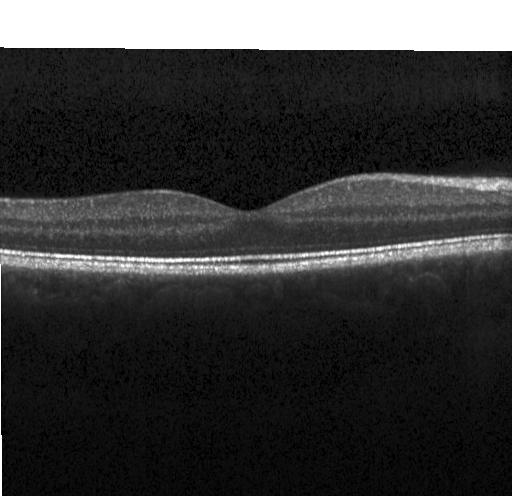 Retinal OCT B-scan, through the macula.
Finding: no choroidal neovascularization, no diabetic macular edema, and no drusen.